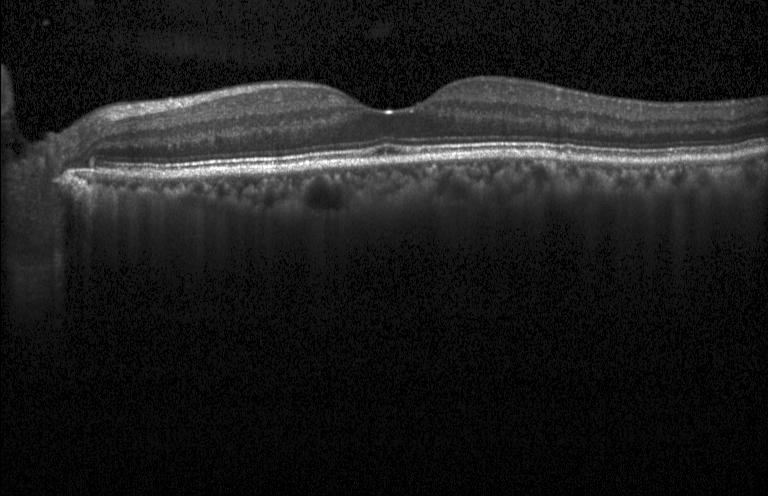
OCT line scan · Heidelberg Spectralis
Impression: no choroidal neovascularization, diabetic macular edema, or drusen.